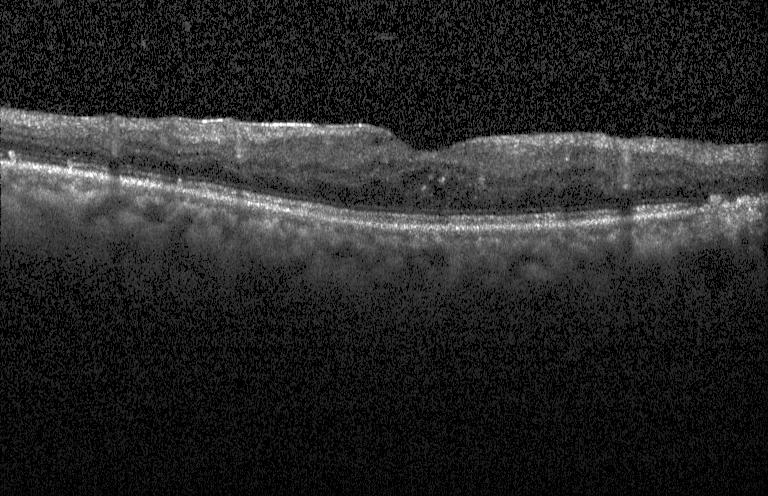

Spectral-domain optical coherence tomography · Heidelberg Spectralis · OCT B-scan · fovea-centered.
The scan shows diabetic macular edema.